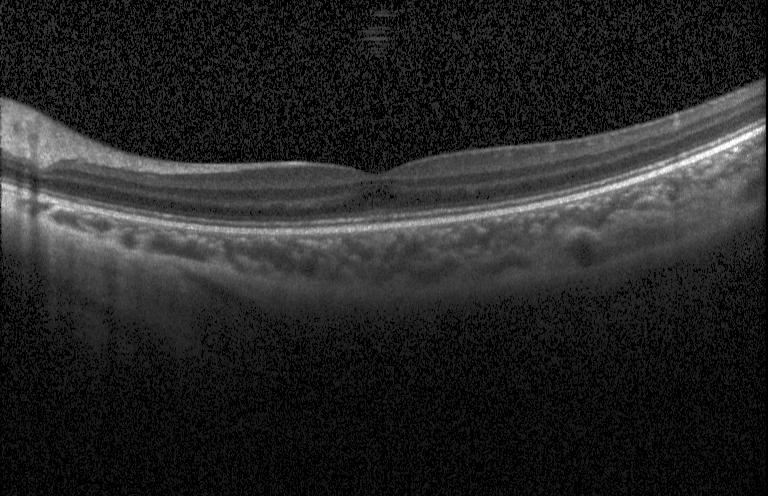 Retinal OCT cross-section — The scan shows no evidence of choroidal neovascularization, diabetic macular edema, or drusen.